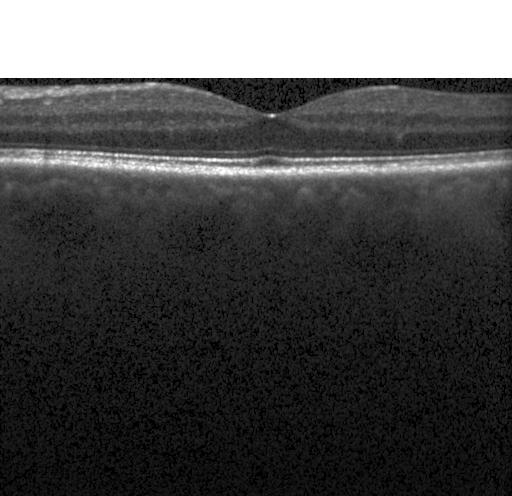
The scan shows no evidence of choroidal neovascularization, diabetic macular edema, or drusen.